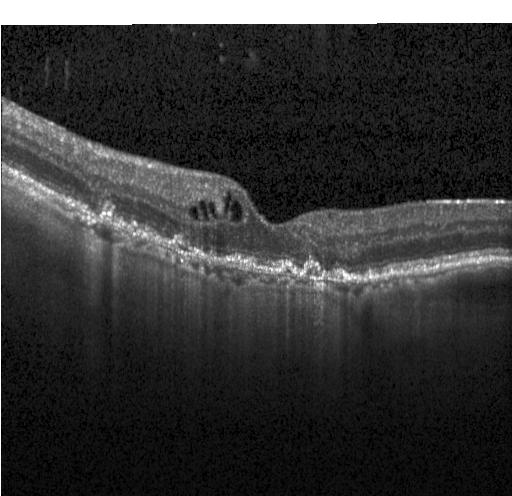 Retinal OCT cross-section · fovea-centered · Heidelberg Spectralis OCT system. Impression: choroidal neovascularization.